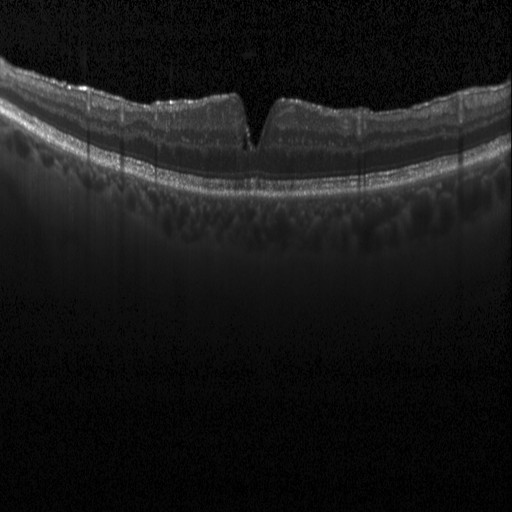

Optical coherence tomography scan, SD-OCT, Heidelberg Spectralis OCT system. The scan shows DME.